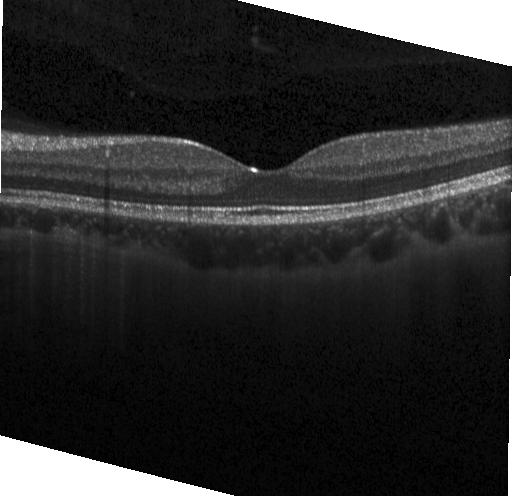
Impression: no choroidal neovascularization, no diabetic macular edema, and no drusen.